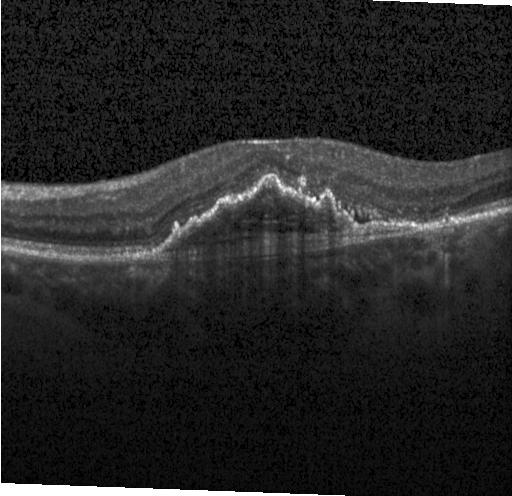 Impression: CNV.